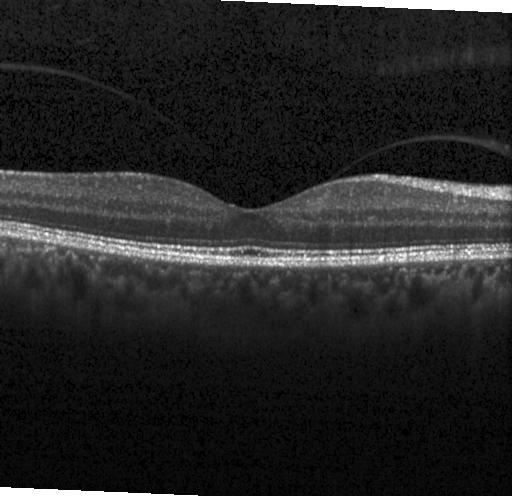

Finding: no choroidal neovascularization, no diabetic macular edema, and no drusen.